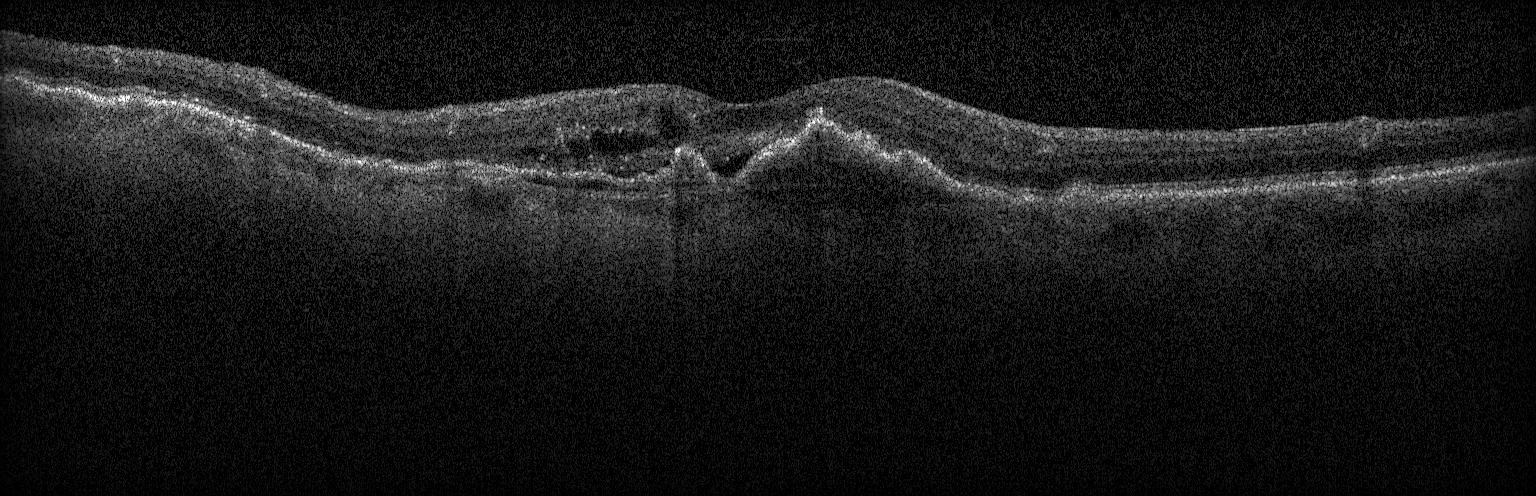 Heidelberg Spectralis · optical coherence tomography scan.
Impression: choroidal neovascularization.